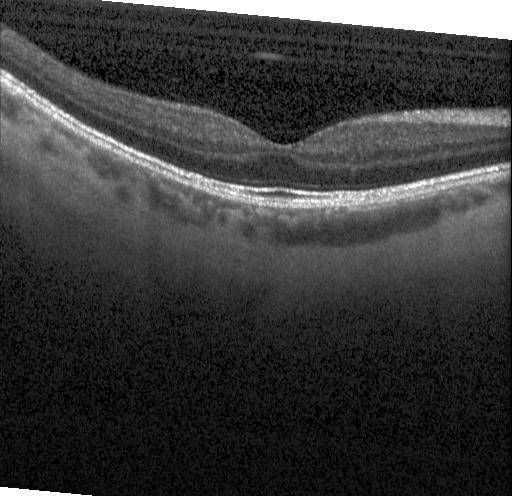 OCT B-scan. No CNV, no DME, and no drusen.